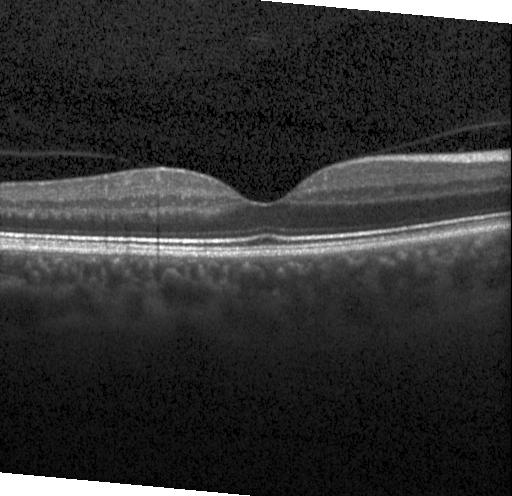

OCT scan showing neither choroidal neovascularization, diabetic macular edema, nor drusen.